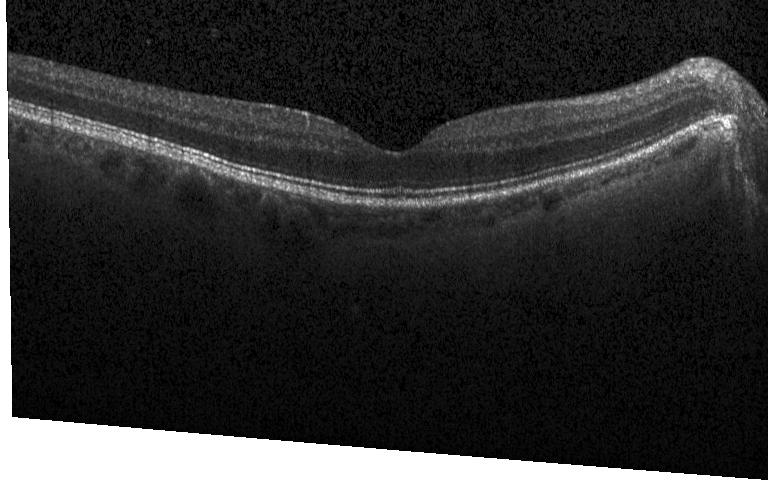 Macular OCT: neither CNV, DME, nor drusen.